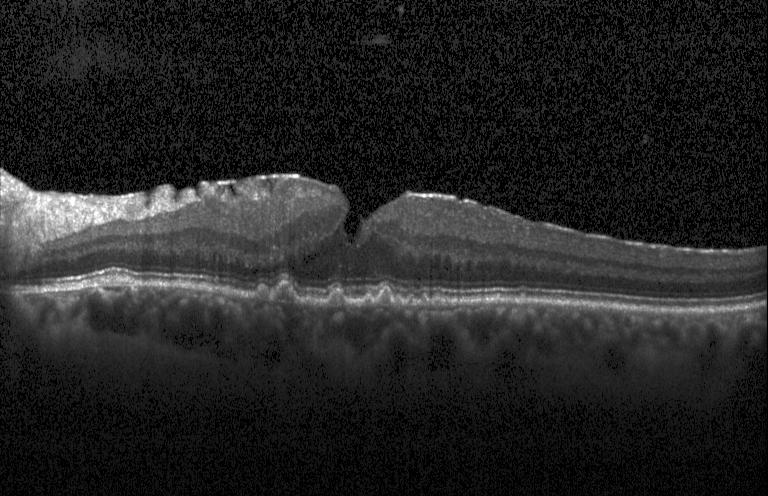

Macular OCT demonstrating multiple drusen.